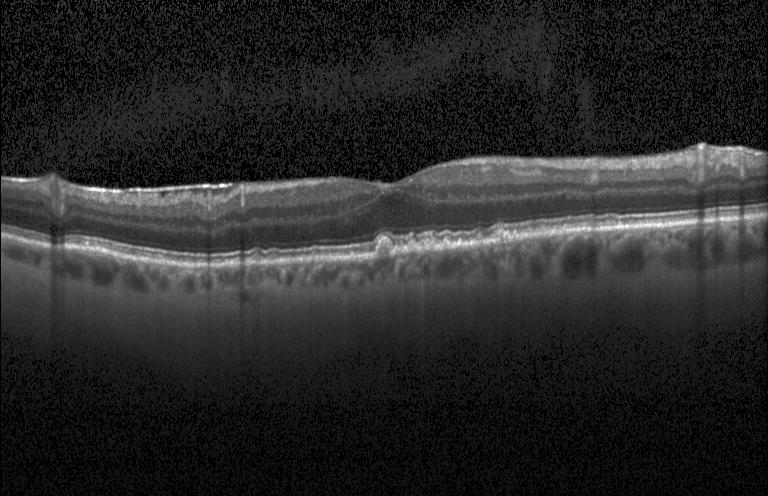
Fovea-centered. Heidelberg Spectralis. Optical coherence tomography B-scan. SD-OCT
Assessment: sub-RPE drusenoid deposits.